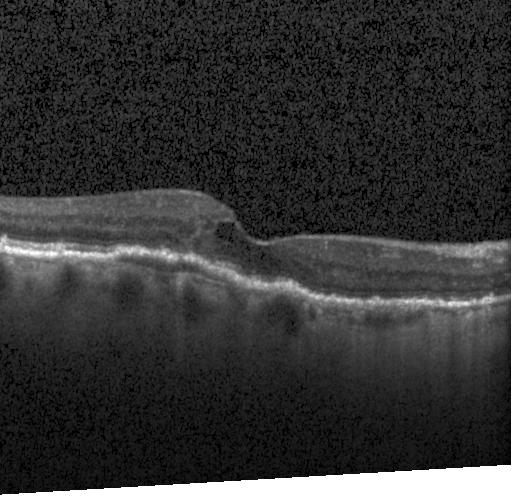

Macular OCT: choroidal neovascularization.